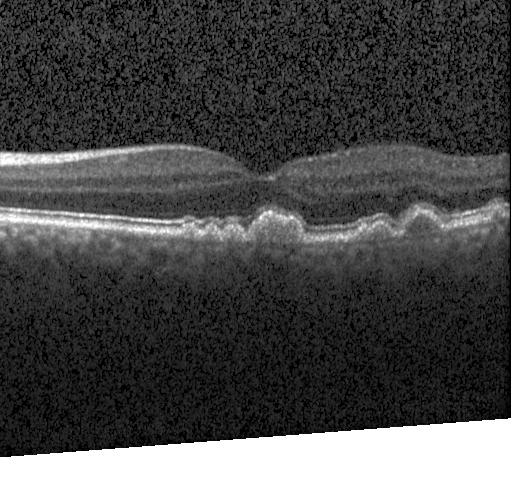 Acquired on a Heidelberg Spectralis, optical coherence tomography B-scan, macular scan — OCT finding: sub-RPE drusenoid deposits.